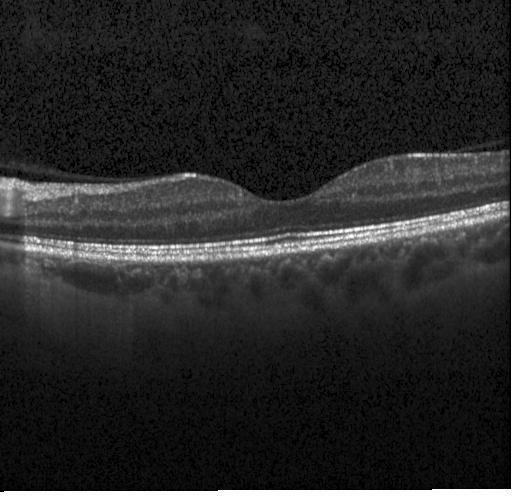 Optical coherence tomography scan. Through the macula. Spectral-domain OCT. Impression: no CNV, DME, or drusen.